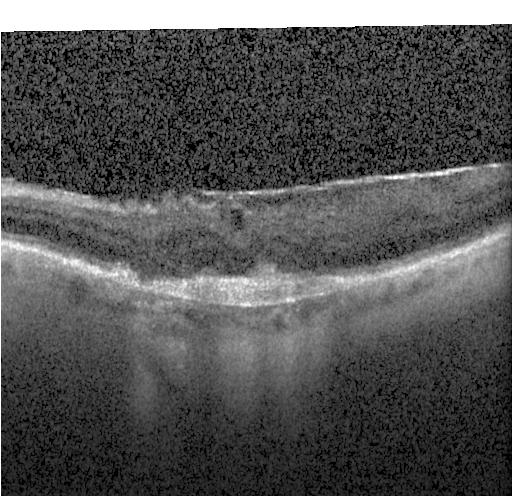
Spectral-domain OCT, through the macula, optical coherence tomography scan.
Impression: a choroidal neovascular membrane.